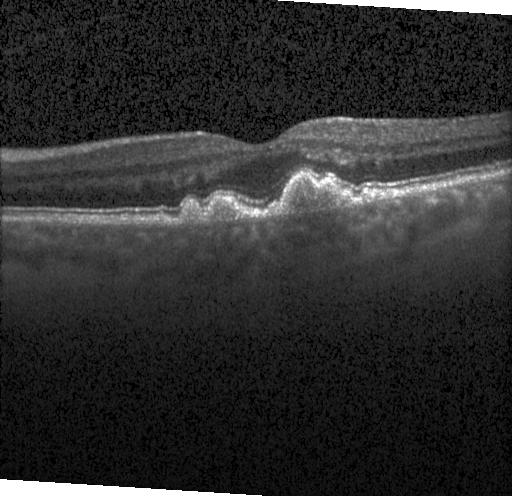 Spectral-domain OCT B-scan: a choroidal neovascular membrane.